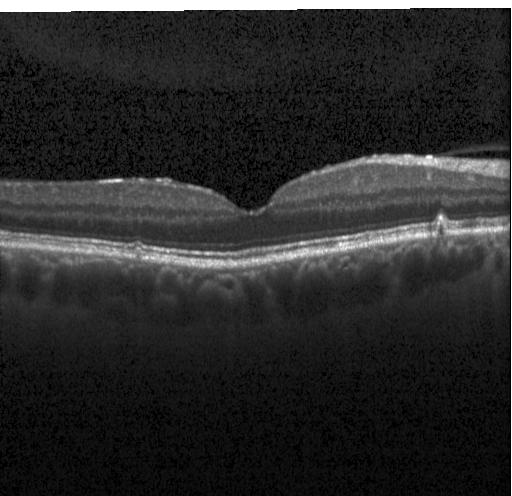

Spectral-domain OCT · OCT B-scan.
This B-scan demonstrates sub-RPE drusenoid deposits.